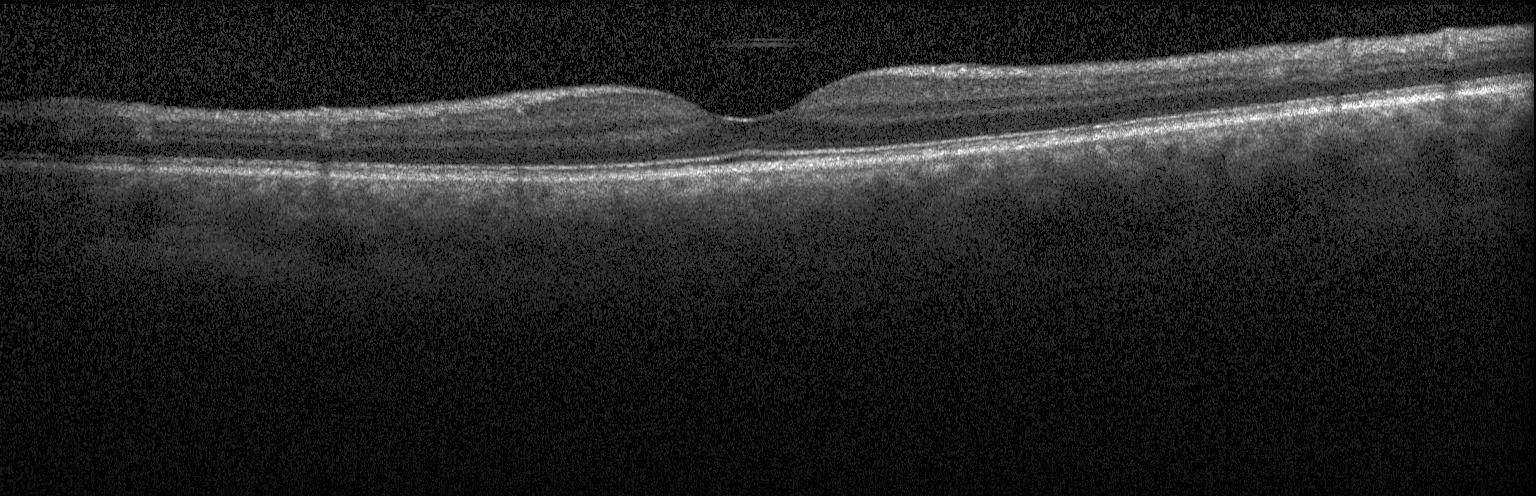

Fovea-centered, retinal OCT B-scan, spectral-domain OCT.
The scan shows neither choroidal neovascularization, diabetic macular edema, nor drusen.